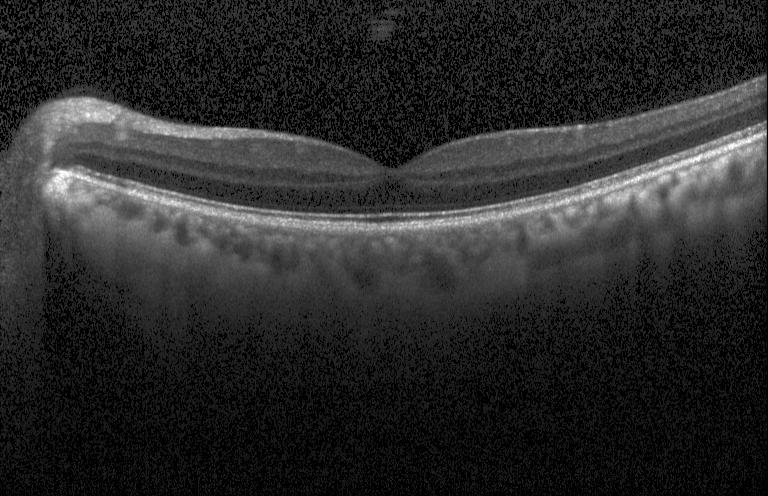
No evidence of choroidal neovascularization, diabetic macular edema, or drusen.